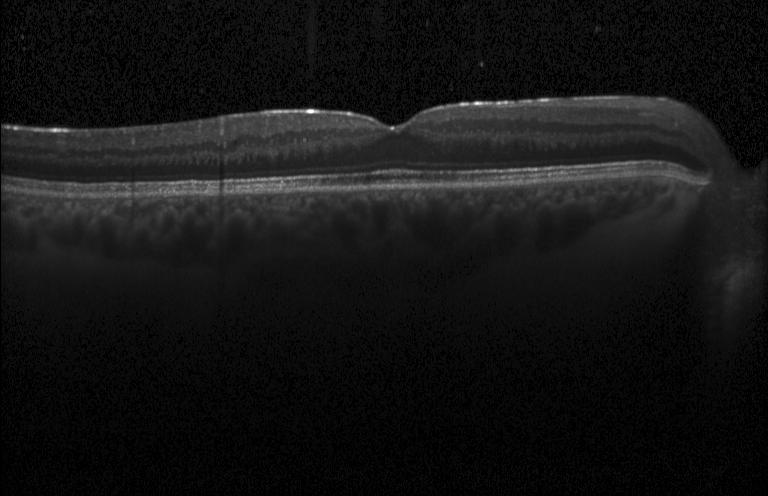
Diagnosis: neither CNV, DME, nor drusen.